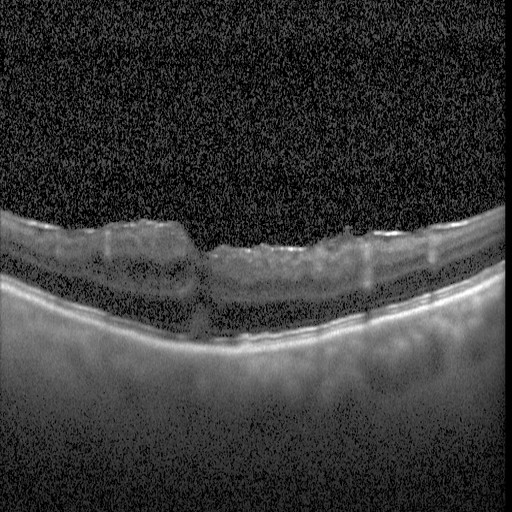 OCT B-scan. Acquired on a Heidelberg Spectralis — OCT finding: DME.